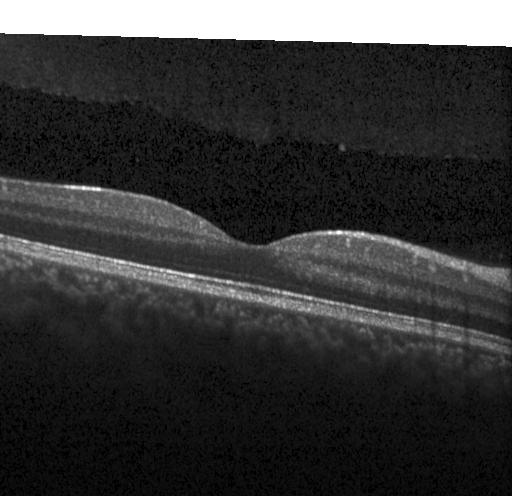 Finding: no evidence of choroidal neovascularization, diabetic macular edema, or drusen.